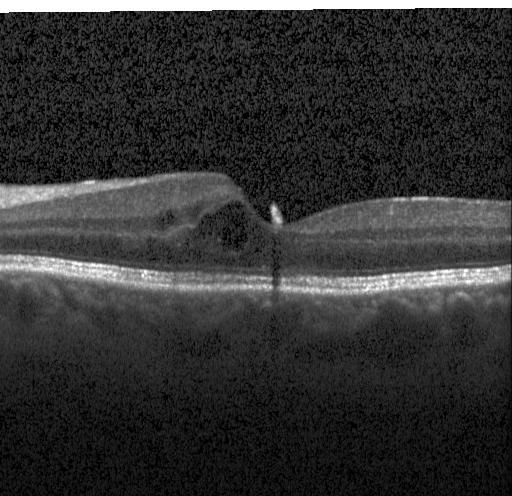

Horizontal scan through the fovea, Heidelberg Spectralis, optical coherence tomography scan.
Diagnosis: DME.